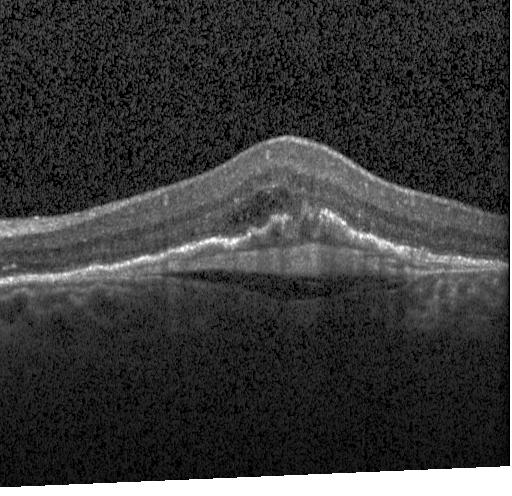

OCT B-scan showing a choroidal neovascular membrane.